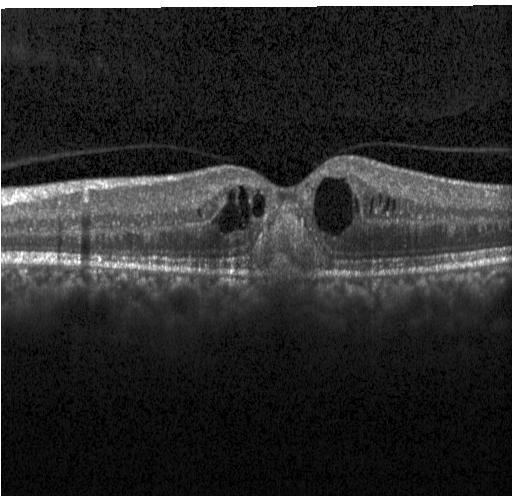 This B-scan demonstrates a choroidal neovascular membrane.